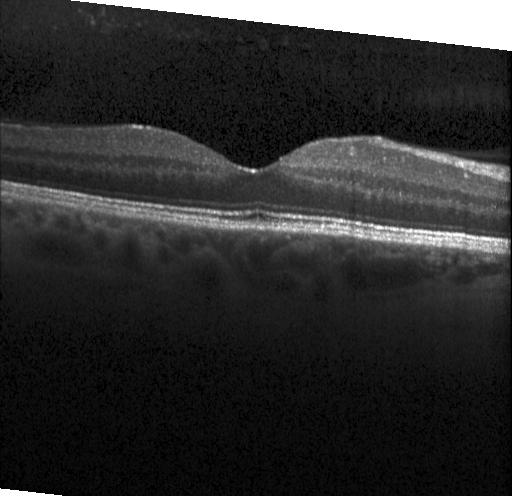 OCT B-scan showing no CNV, DME, or drusen.